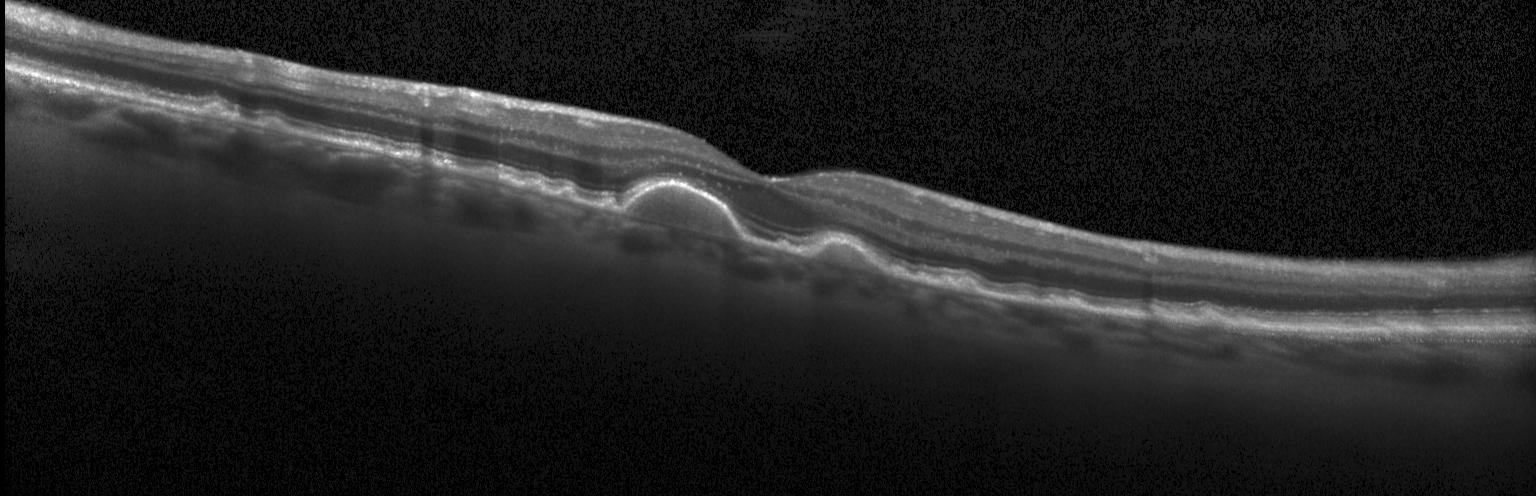
The scan shows multiple drusen.